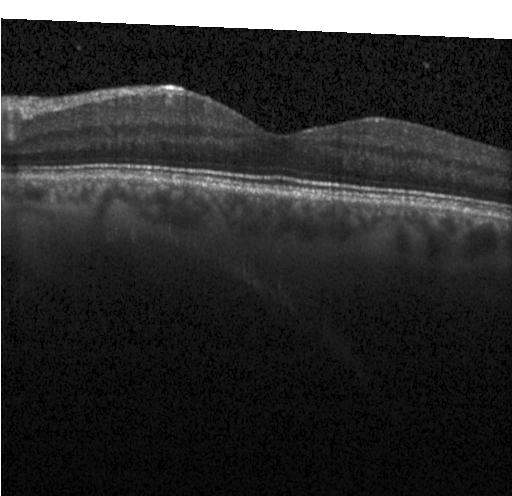

OCT B-scan. Instrument: Heidelberg Spectralis.
Impression: no choroidal neovascularization, diabetic macular edema, or drusen.